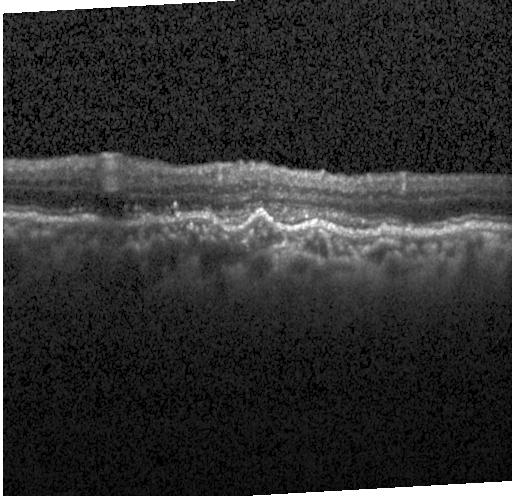
Diagnosis: a choroidal neovascular membrane.